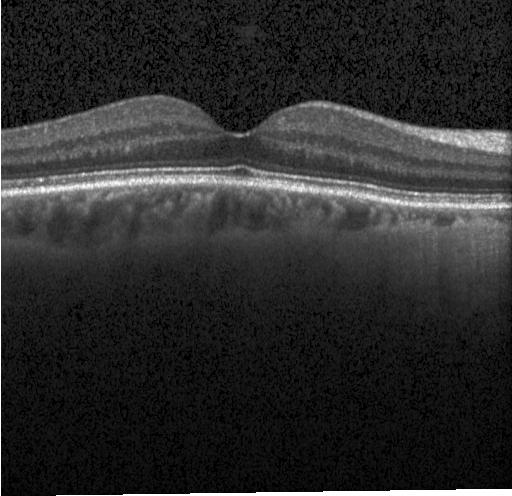

Impression: no CNV, no DME, and no drusen.